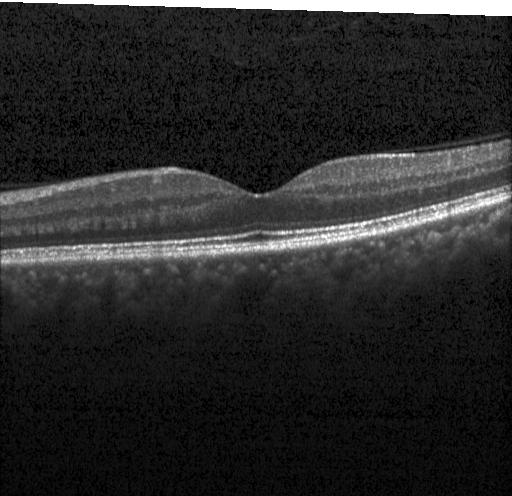

OCT scan showing no evidence of CNV, DME, or drusen.